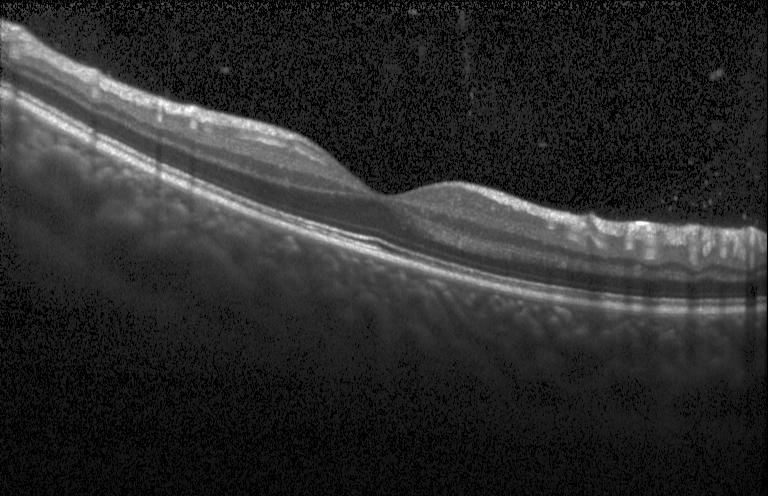

Optical coherence tomography B-scan · Heidelberg Spectralis — Dx: no evidence of choroidal neovascularization, diabetic macular edema, or drusen.